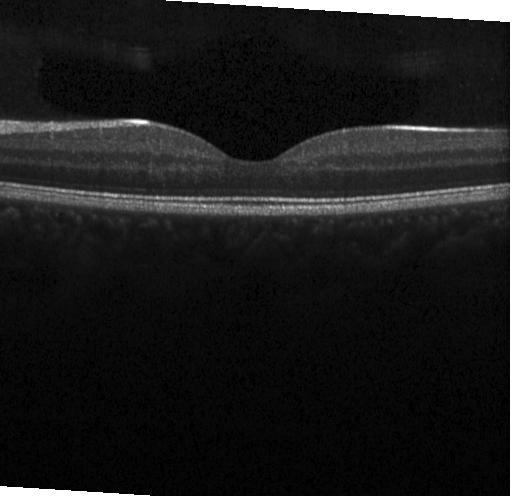 OCT B-scan showing neither choroidal neovascularization, diabetic macular edema, nor drusen.